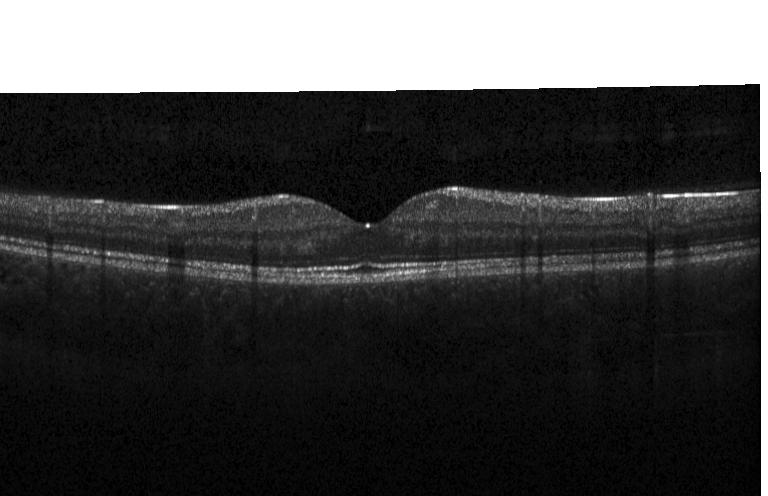 Retinal OCT cross-section · centered on the fovea · Heidelberg Spectralis OCT system · spectral-domain OCT — Diagnosis: no evidence of choroidal neovascularization, diabetic macular edema, or drusen.